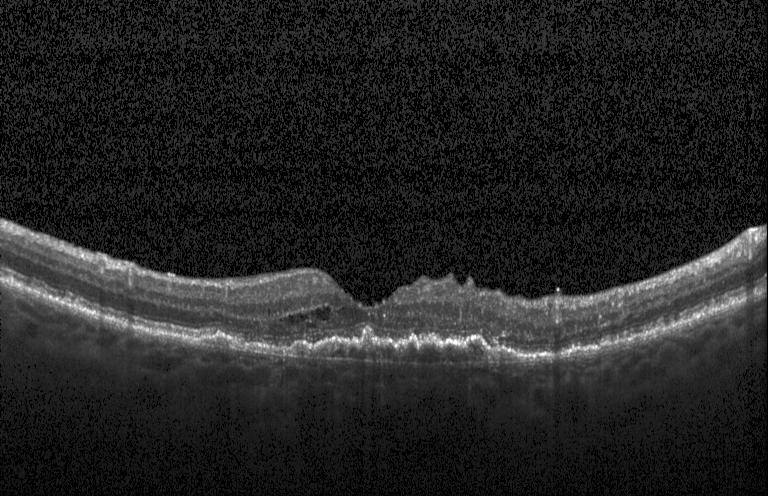 A choroidal neovascular membrane.